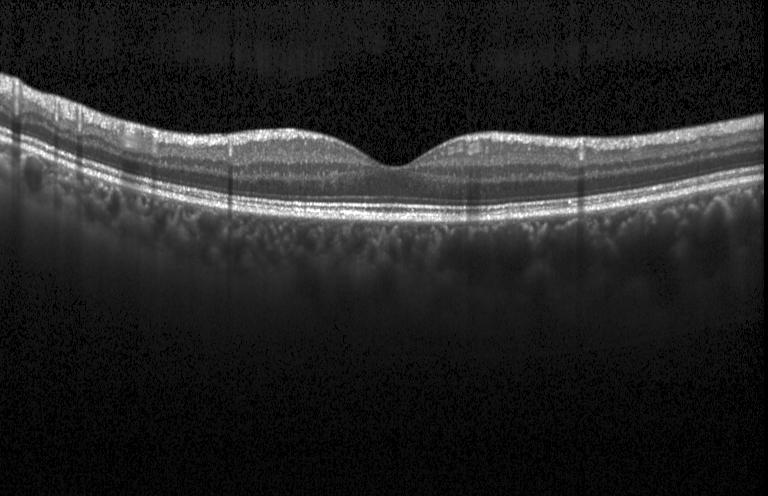

Diagnosis: no evidence of choroidal neovascularization, diabetic macular edema, or drusen.